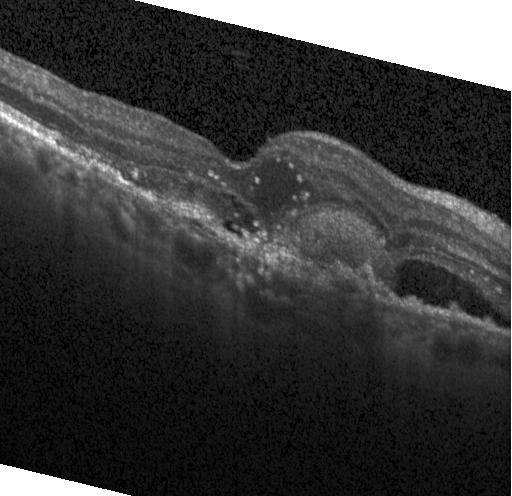 Retinal OCT cross-section, acquired on a Heidelberg Spectralis.
This B-scan demonstrates choroidal neovascularization (CNV).